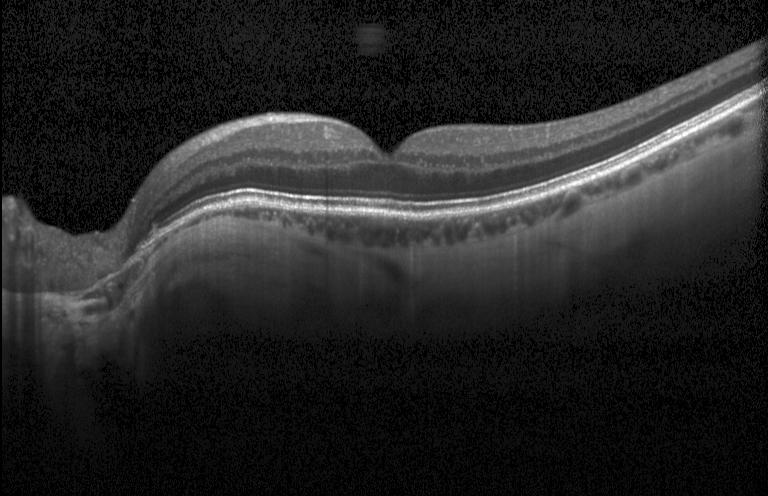

Retinal OCT B-scan. Spectral-domain optical coherence tomography.
Macular OCT: no evidence of choroidal neovascularization, diabetic macular edema, or drusen.